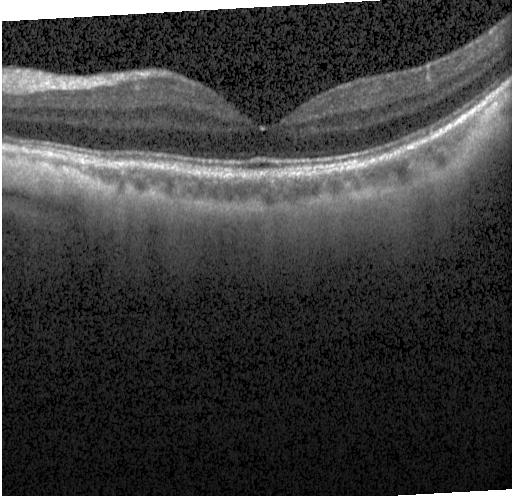

Optical coherence tomography scan, spectral-domain OCT
This B-scan demonstrates neither choroidal neovascularization, diabetic macular edema, nor drusen.